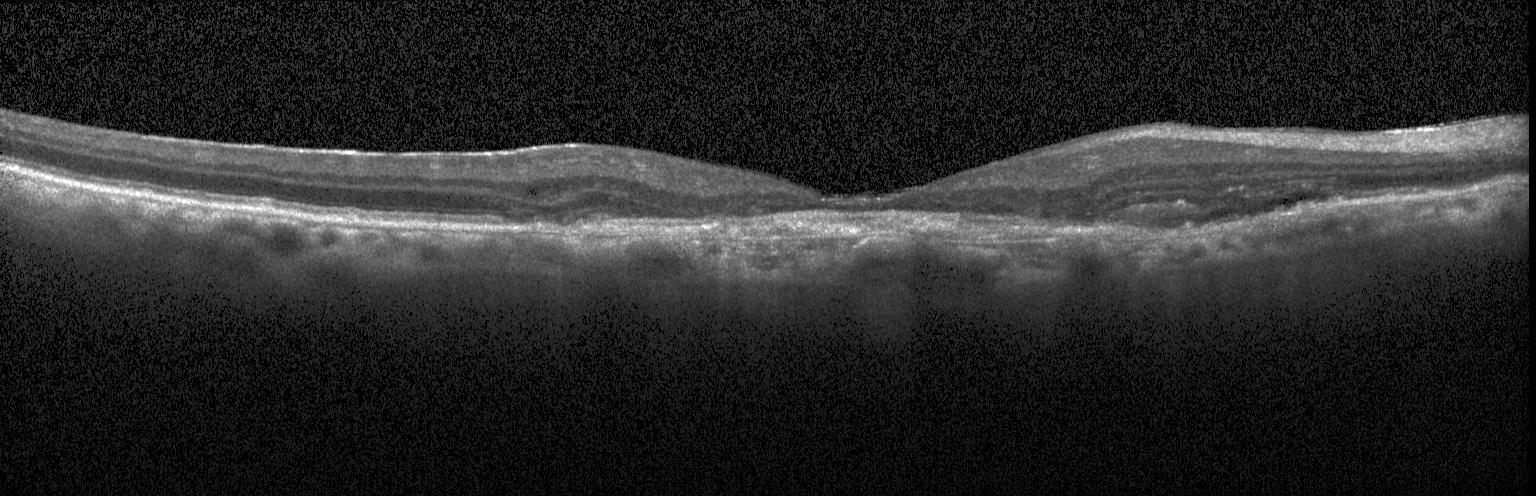 Retinal OCT B-scan. The scan shows CNV.